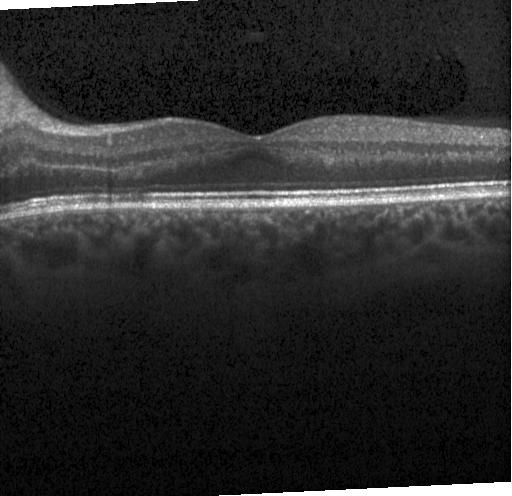

Acquired on a Heidelberg Spectralis; through the macula; OCT B-scan; spectral-domain OCT.
Impression: no CNV, no DME, and no drusen.